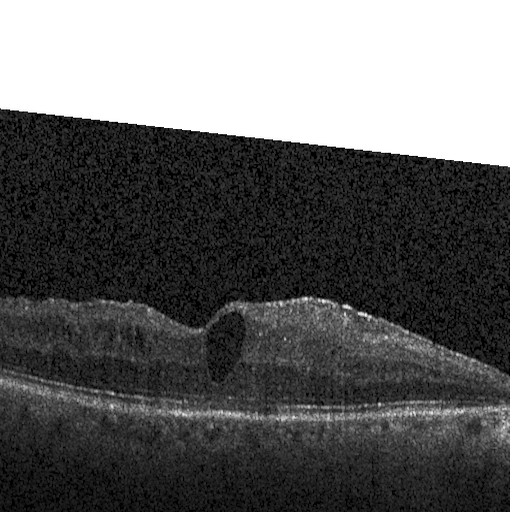
Through the macula. OCT B-scan — Assessment: diabetic macular edema.